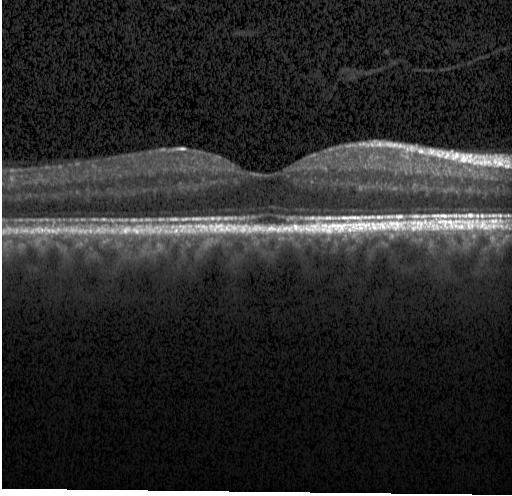
OCT line scan, SD-OCT, fovea-centered, instrument: Heidelberg Spectralis — Diagnosis: no choroidal neovascularization, no diabetic macular edema, and no drusen.